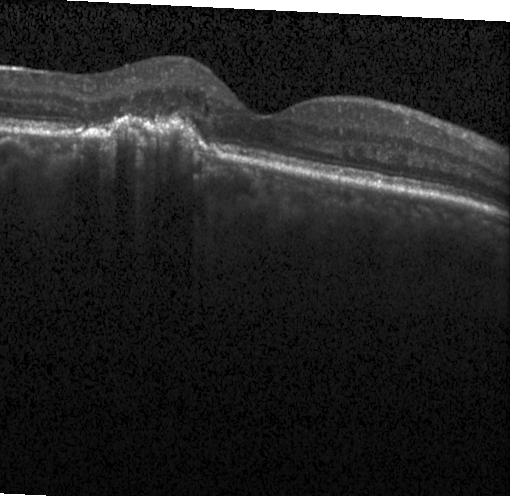 Assessment: choroidal neovascularization (CNV).